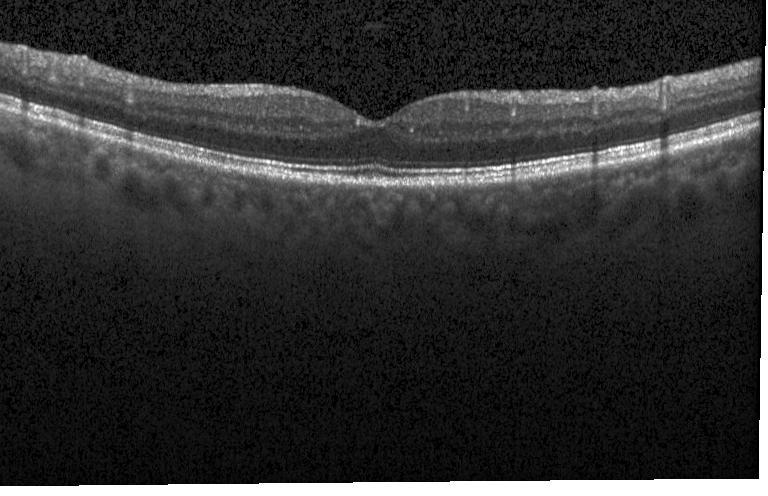 OCT B-scan.
Impression: no evidence of choroidal neovascularization, diabetic macular edema, or drusen.